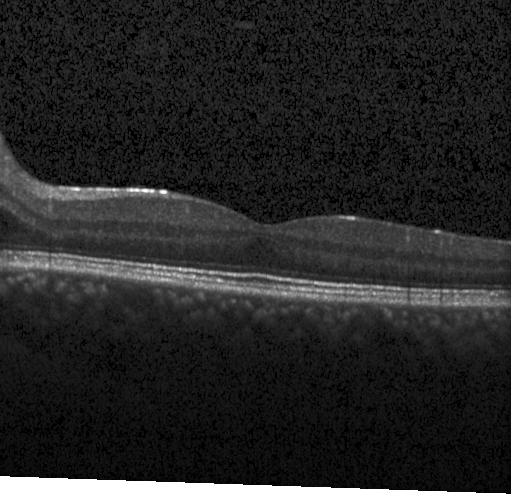

Retinal OCT cross-section showing neither CNV, DME, nor drusen.